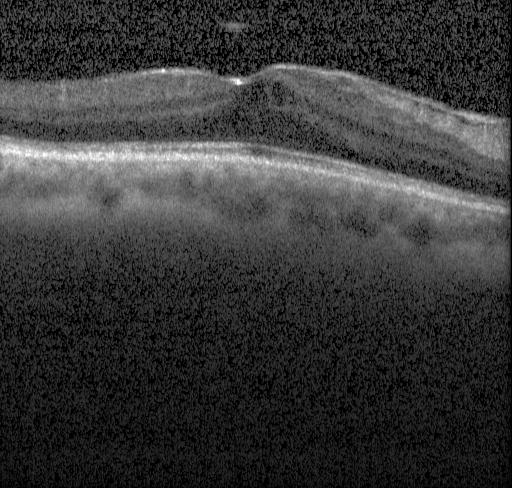
Instrument: Heidelberg Spectralis, retinal OCT B-scan, SD-OCT.
Assessment: diabetic macular edema (DME).